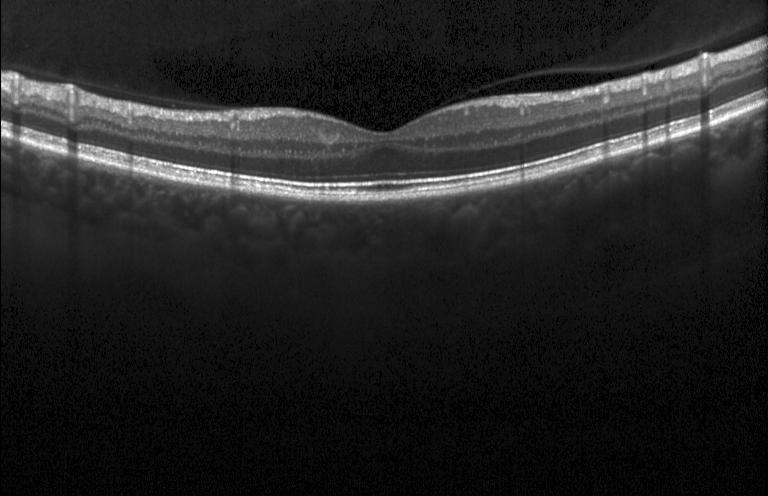
Retinal OCT B-scan — This B-scan demonstrates neither CNV, DME, nor drusen.